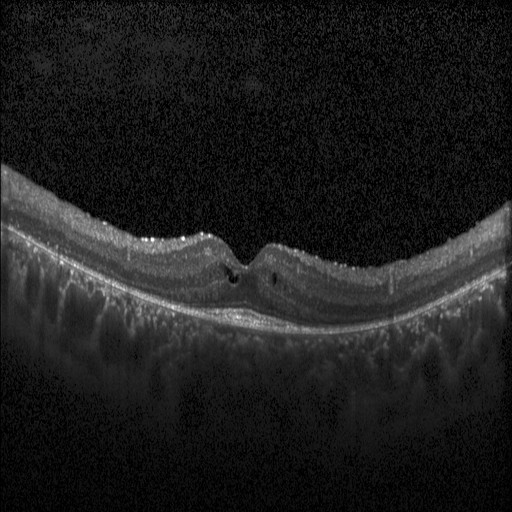
Impression: diabetic macular edema (DME).